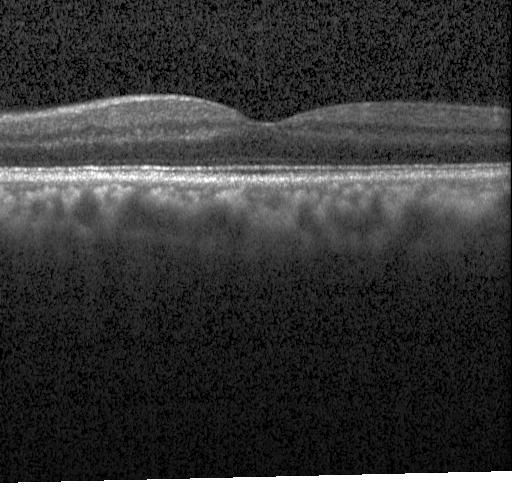

The scan shows neither CNV, DME, nor drusen.